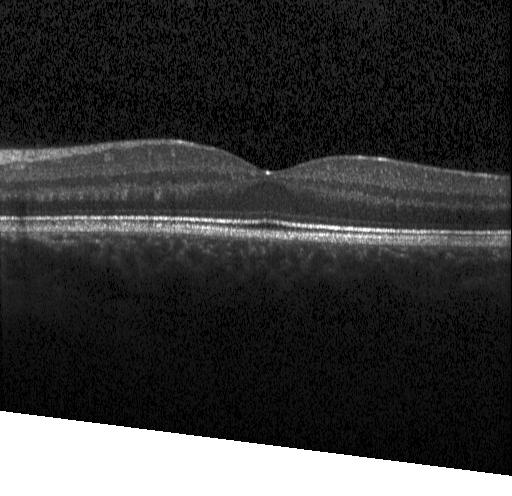
Retinal OCT B-scan.
No evidence of choroidal neovascularization, diabetic macular edema, or drusen.